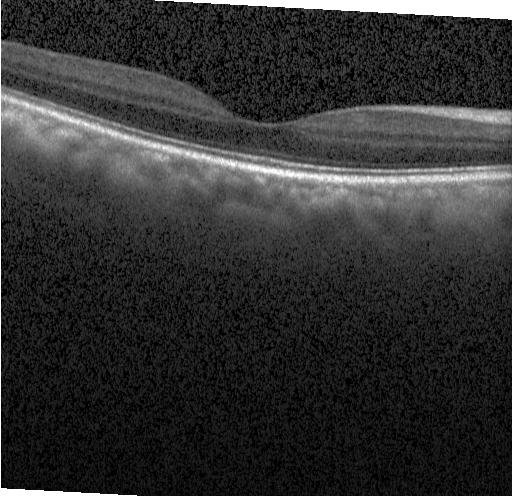

This B-scan demonstrates neither choroidal neovascularization, diabetic macular edema, nor drusen.